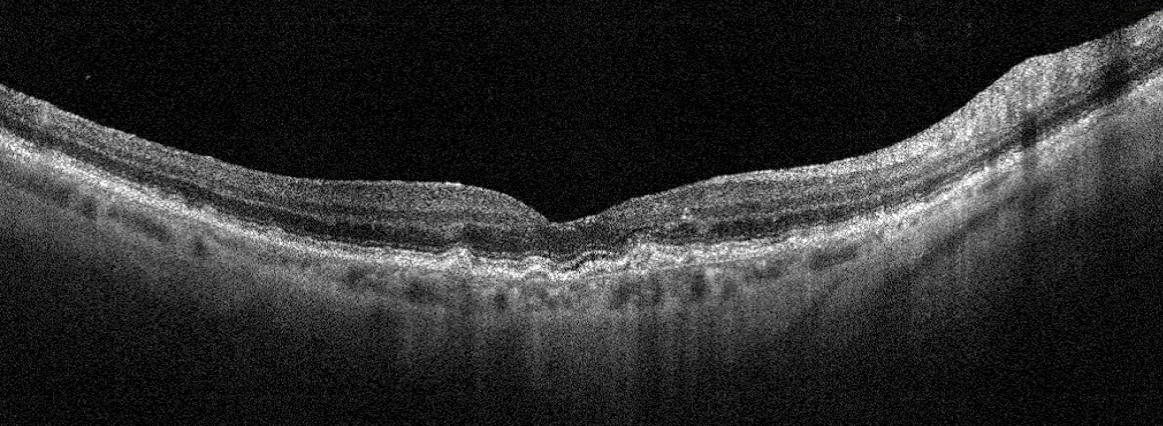 Oculus dexter · retinal OCT cross-section.
OCT finding: age-related macular degeneration.